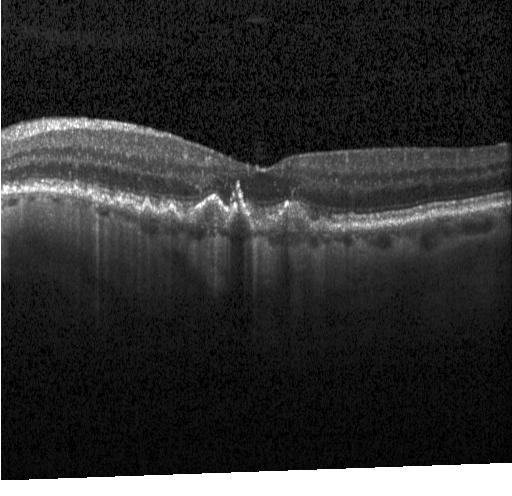 Instrument: Heidelberg Spectralis · SD-OCT · retinal OCT B-scan.
OCT finding: multiple drusen.